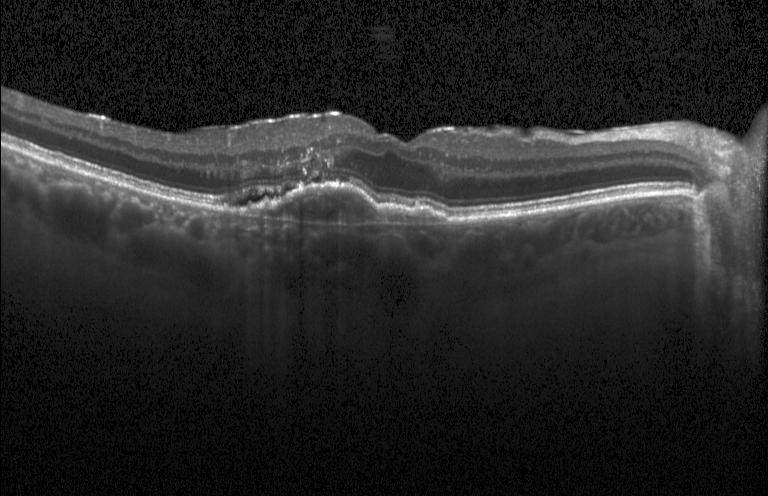

Optical coherence tomography B-scan · instrument: Heidelberg Spectralis.
This B-scan demonstrates a choroidal neovascular membrane.